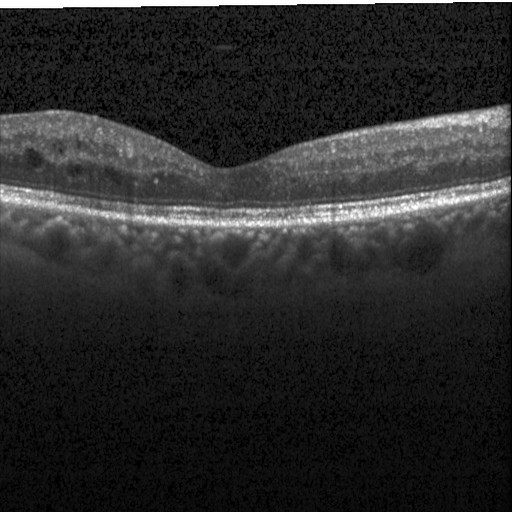 Finding: DME.